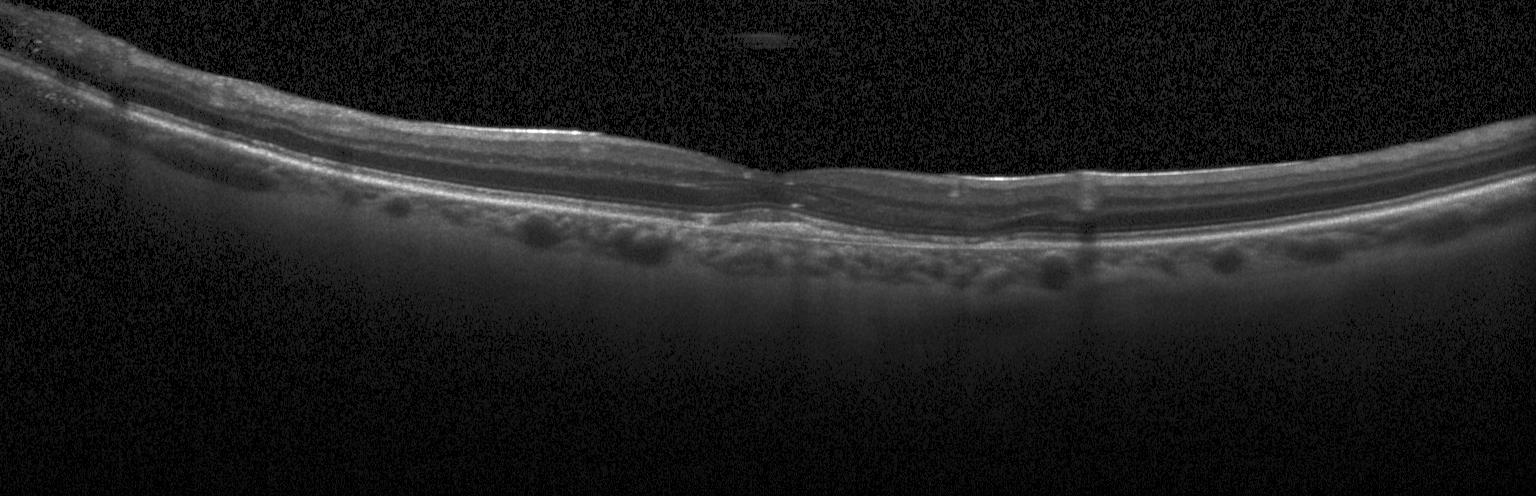

Centered on the fovea, retinal OCT B-scan, acquired on a Heidelberg Spectralis.
Impression: a choroidal neovascular membrane.